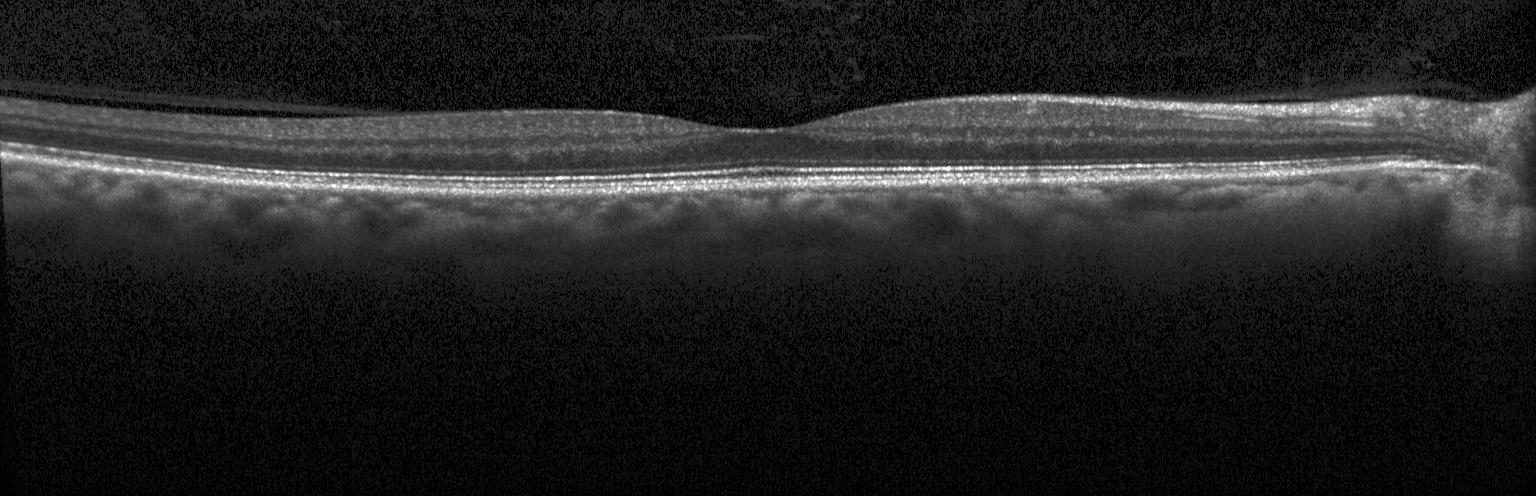 Optical coherence tomography B-scan · fovea-centered · acquired on a Heidelberg Spectralis — Finding: no choroidal neovascularization, no diabetic macular edema, and no drusen.